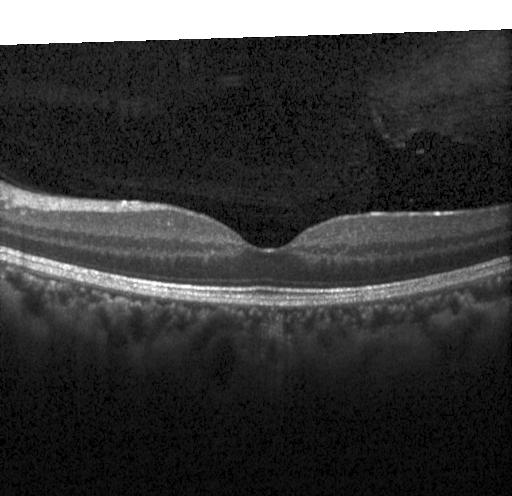 Retinal OCT cross-section showing no choroidal neovascularization, diabetic macular edema, or drusen.